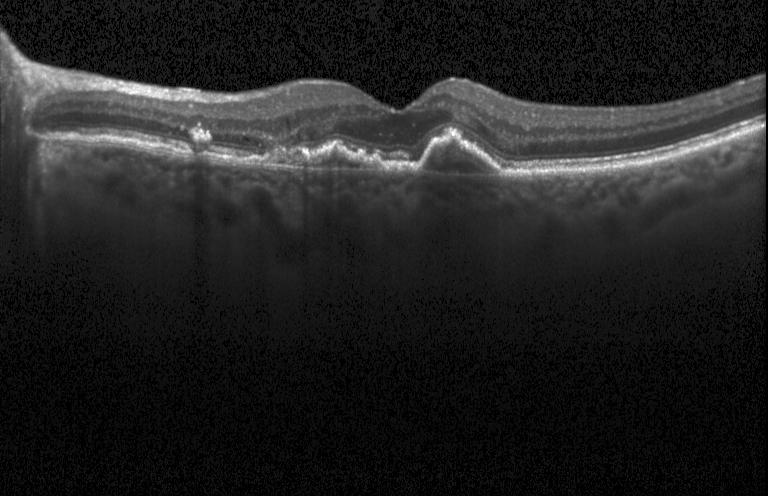
Optical coherence tomography B-scan — Diagnosis: a choroidal neovascular membrane.